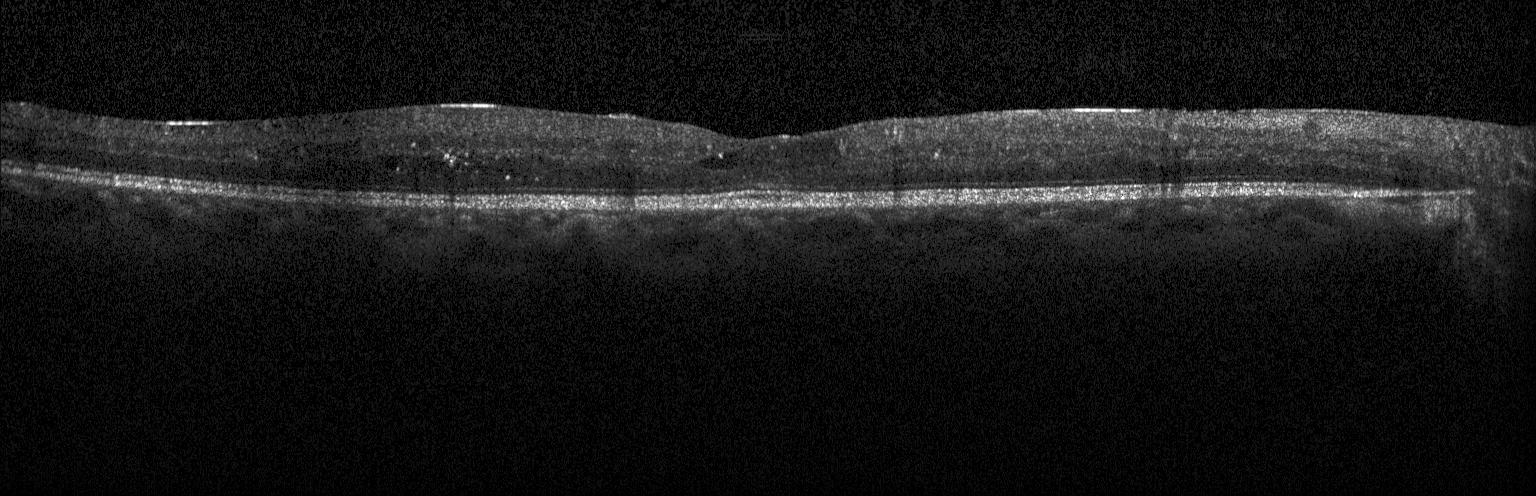
Optical coherence tomography scan; horizontal scan through the fovea.
Macular OCT: DME.